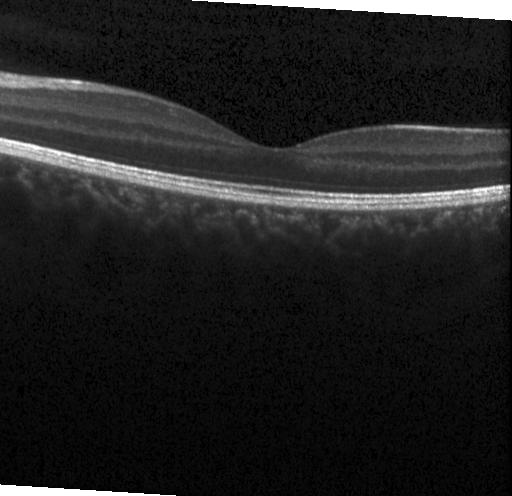 Retinal OCT cross-section. Instrument: Heidelberg Spectralis. Spectral-domain OCT. Fovea-centered — Assessment: no choroidal neovascularization, diabetic macular edema, or drusen.